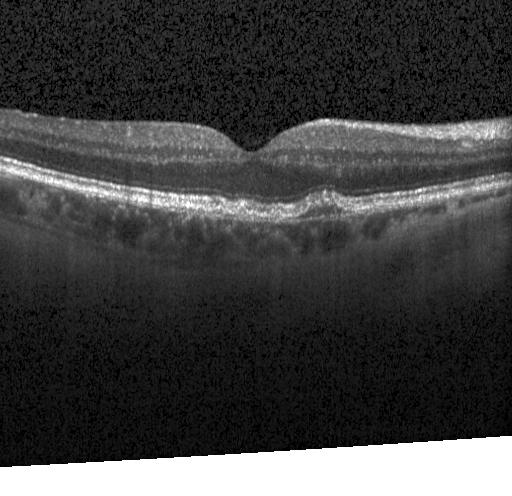

Horizontal scan through the fovea, OCT line scan, SD-OCT — Finding: multiple drusen.